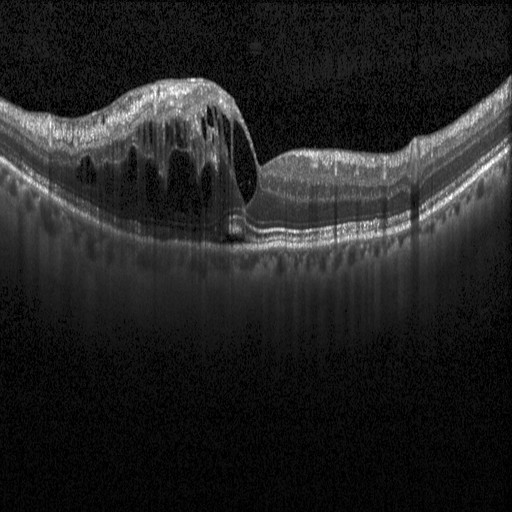 The scan shows diabetic macular edema.